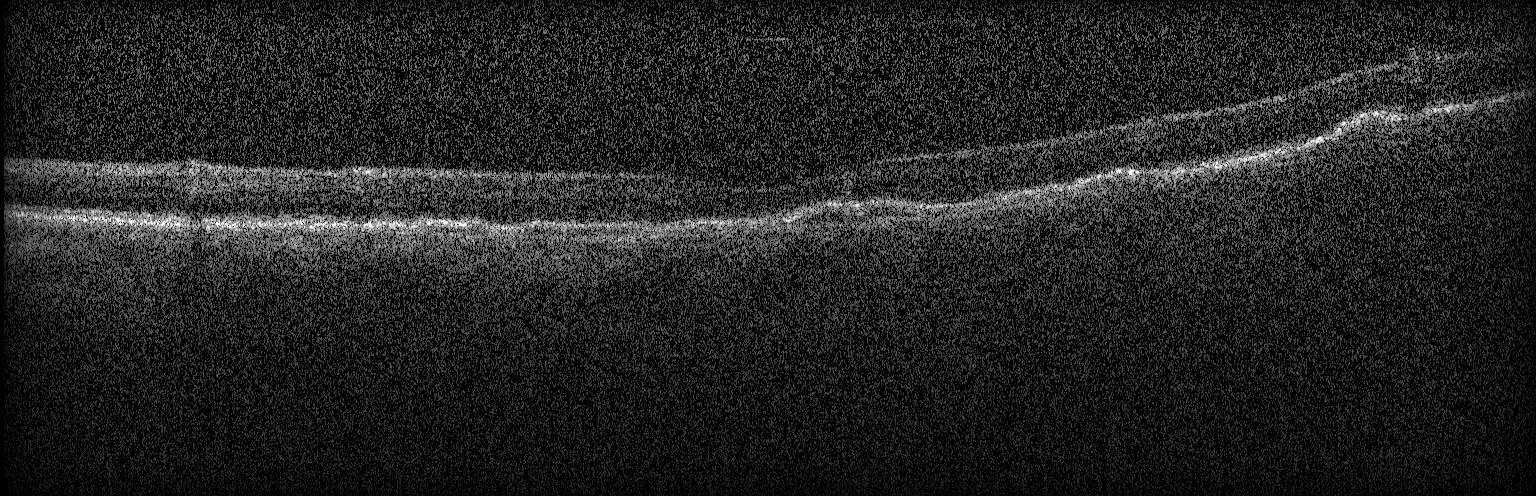

Horizontal scan through the fovea; retinal OCT B-scan; instrument: Heidelberg Spectralis; spectral-domain OCT.
Finding: choroidal neovascularization (CNV).